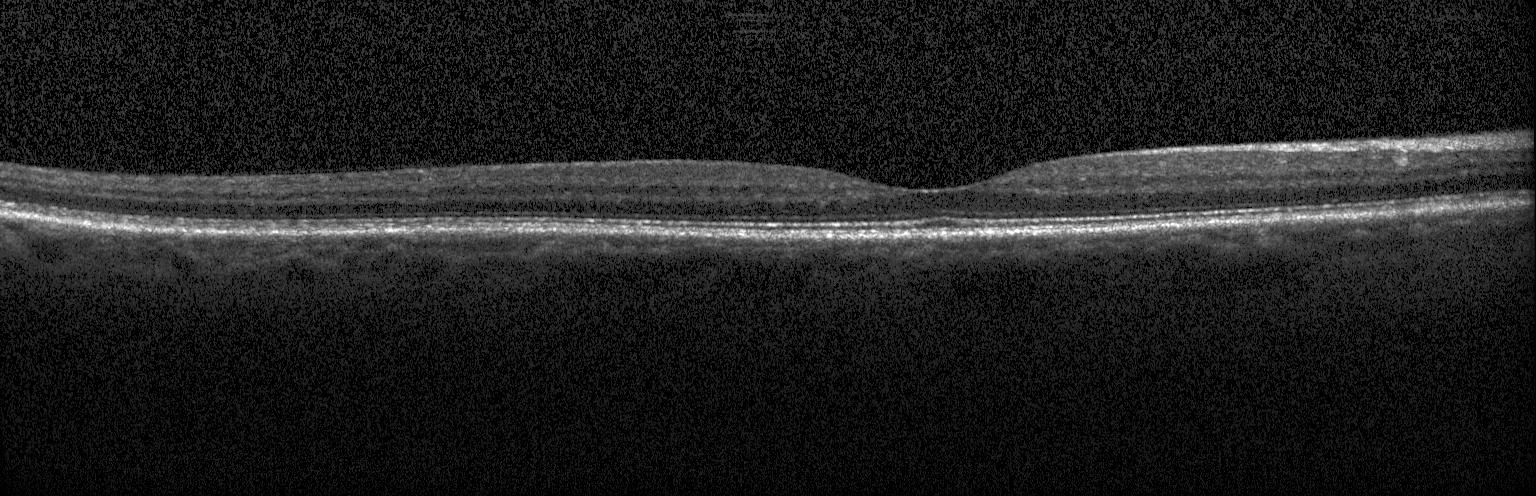
Assessment: no choroidal neovascularization, diabetic macular edema, or drusen.